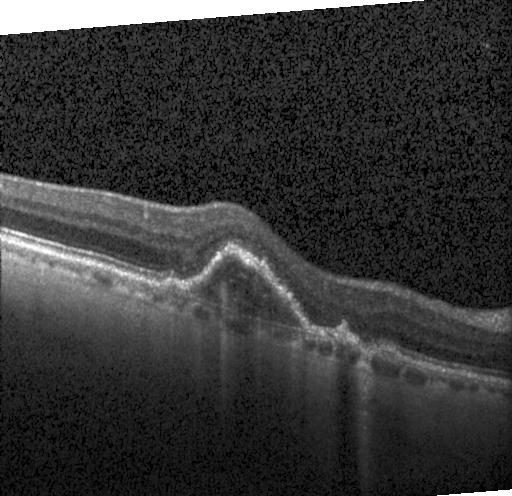 Macular scan. Retinal OCT B-scan — Finding: CNV.